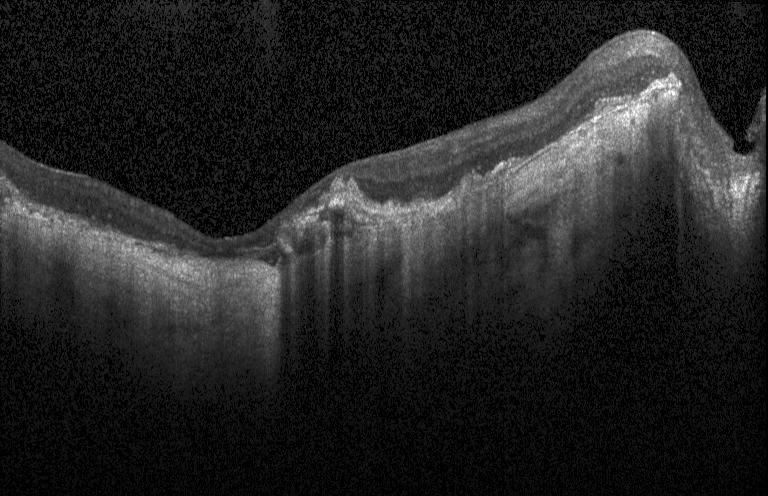
Dx: a choroidal neovascular membrane.